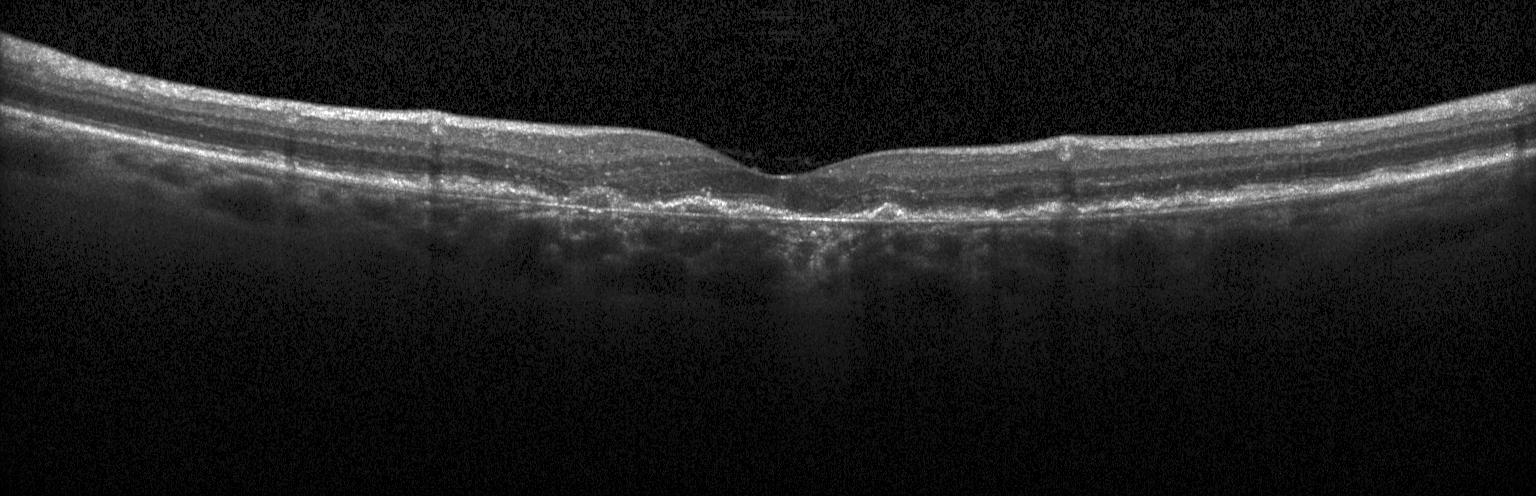 Heidelberg Spectralis; horizontal scan through the fovea; spectral-domain optical coherence tomography; retinal OCT cross-section — Macular OCT: a choroidal neovascular membrane.